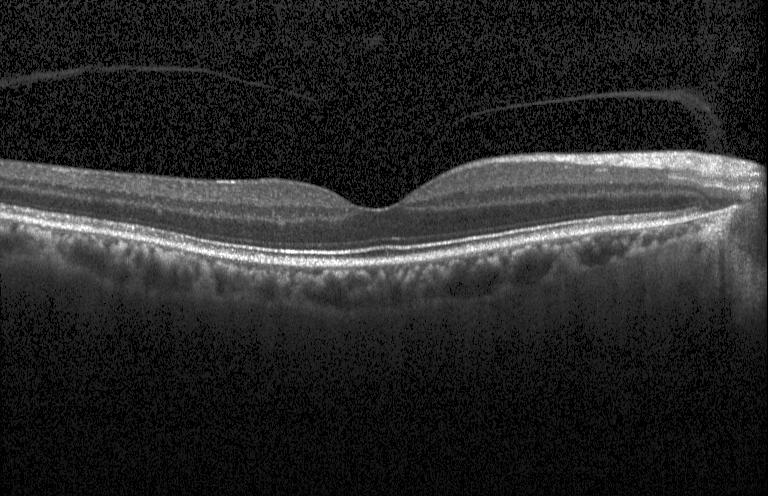
Dx: neither choroidal neovascularization, diabetic macular edema, nor drusen.